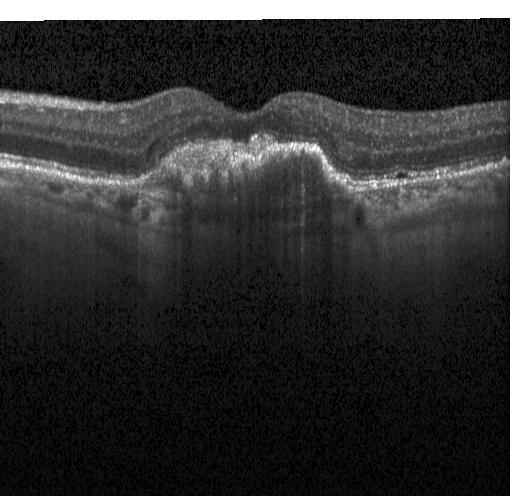
This B-scan demonstrates choroidal neovascularization.